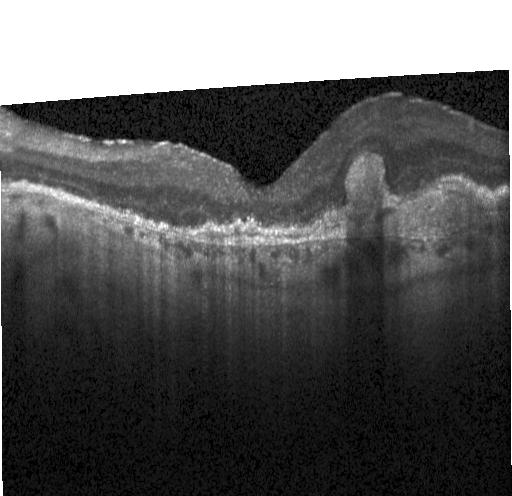 Heidelberg Spectralis OCT system. Optical coherence tomography B-scan — This B-scan demonstrates a choroidal neovascular membrane.